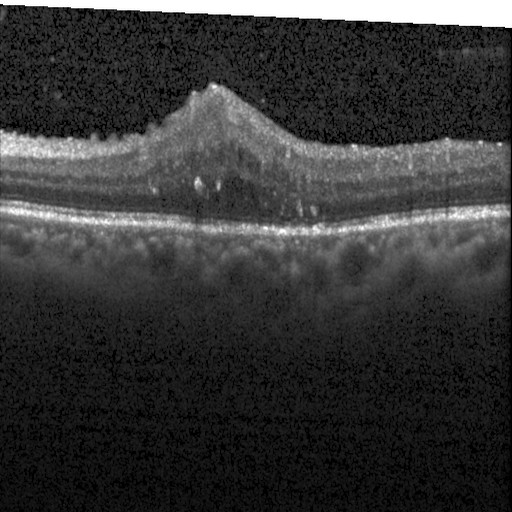 Optical coherence tomography scan; spectral-domain optical coherence tomography.
Finding: diabetic macular edema (DME).